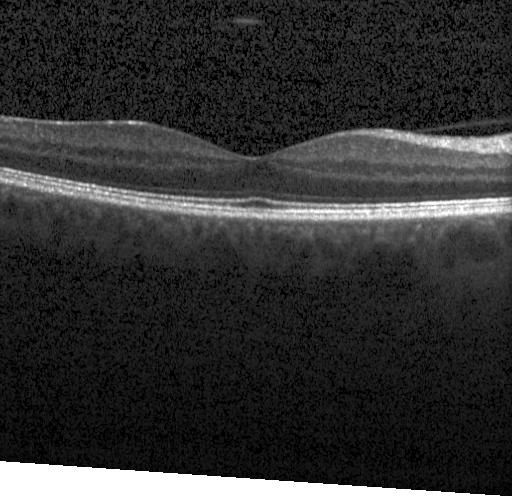

Impression: no choroidal neovascularization, no diabetic macular edema, and no drusen.